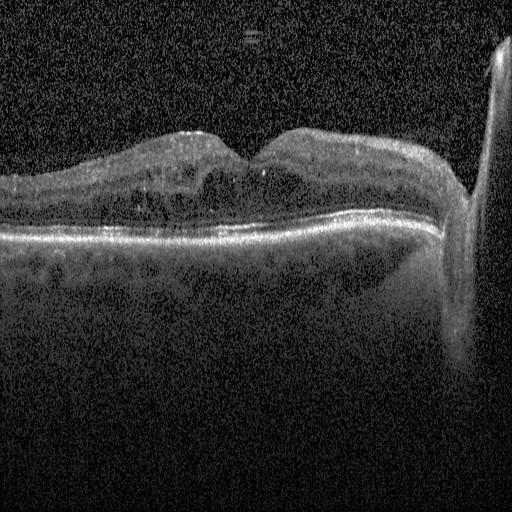
Finding: DME.